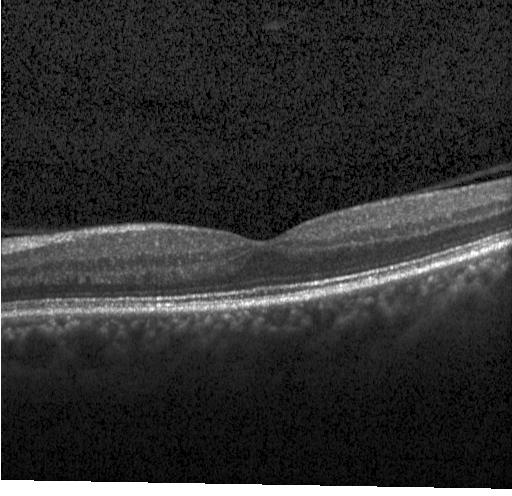

Retinal OCT cross-section
The scan shows no choroidal neovascularization, no diabetic macular edema, and no drusen.